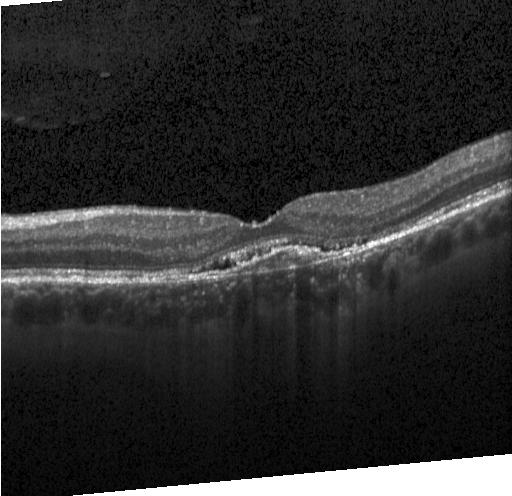
Retinal OCT B-scan; centered on the fovea
Dx: choroidal neovascularization (CNV).